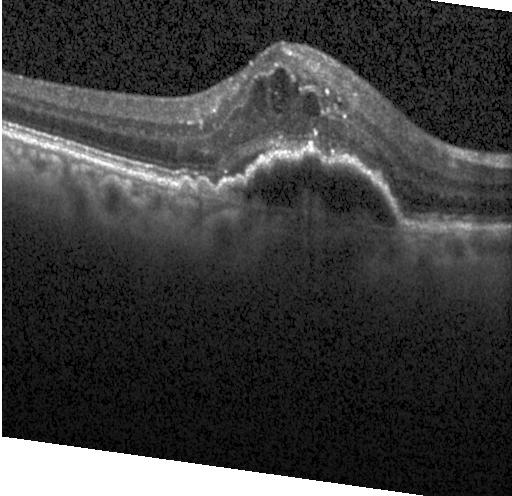

Choroidal neovascularization.